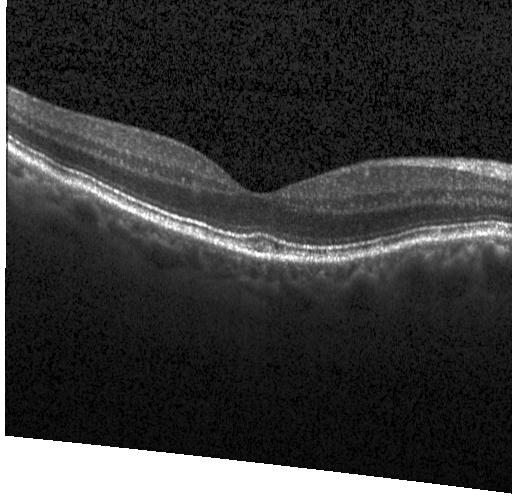
Finding: neither choroidal neovascularization, diabetic macular edema, nor drusen.